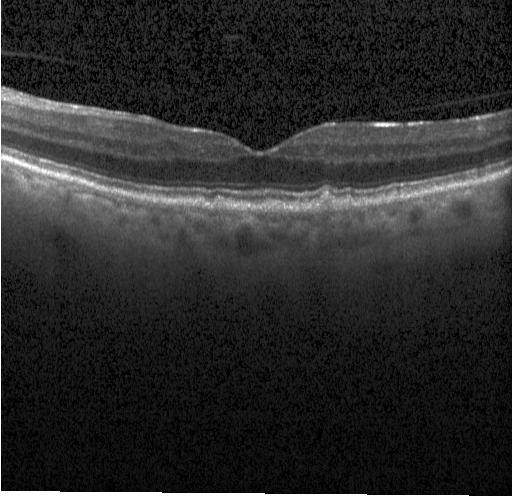
Heidelberg Spectralis · retinal OCT B-scan · through the macula
Impression: multiple drusen.